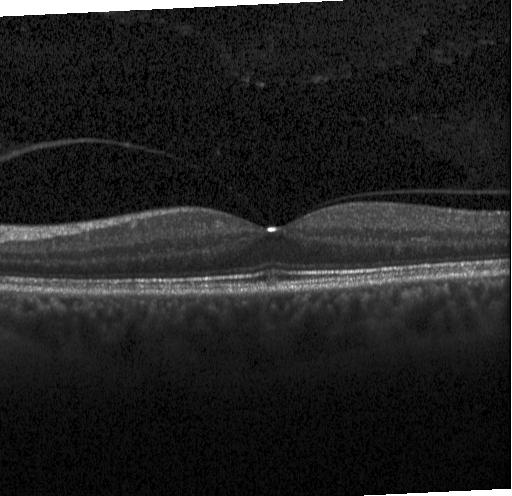 Finding: no choroidal neovascularization, no diabetic macular edema, and no drusen.